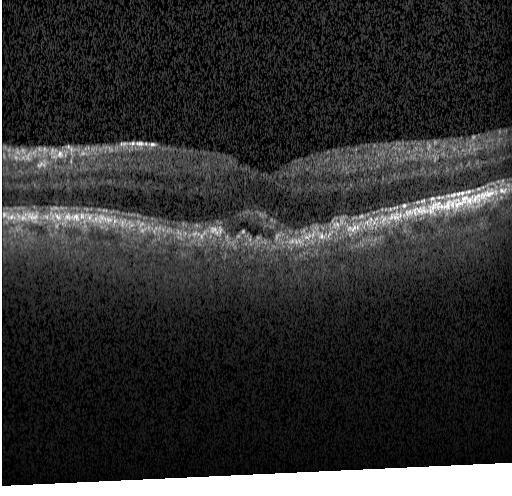 OCT line scan. A choroidal neovascular membrane.